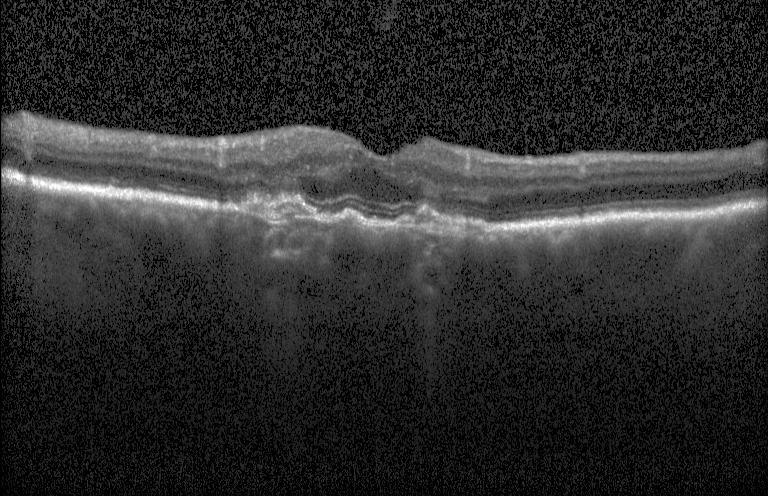

Finding: choroidal neovascularization.